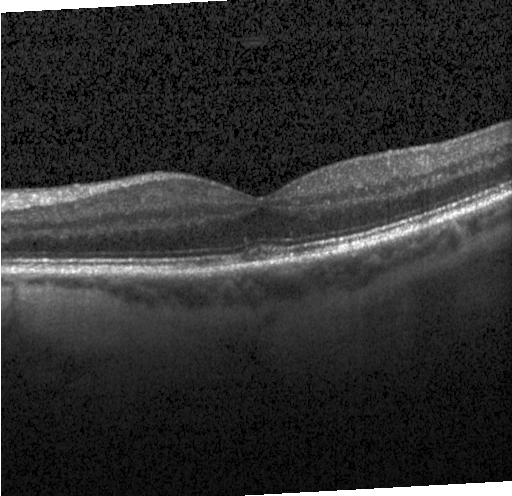 OCT B-scan showing no evidence of CNV, DME, or drusen.